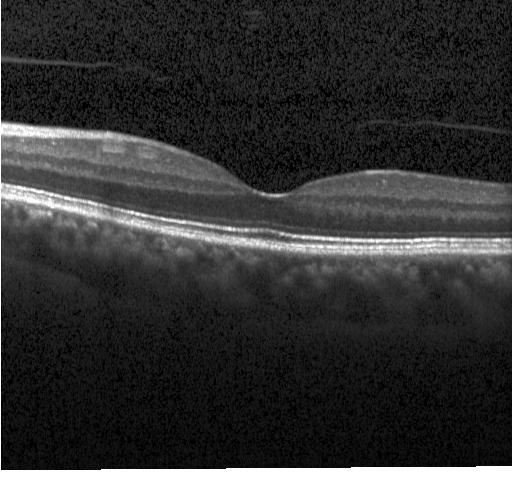
Macular OCT: no evidence of choroidal neovascularization, diabetic macular edema, or drusen.